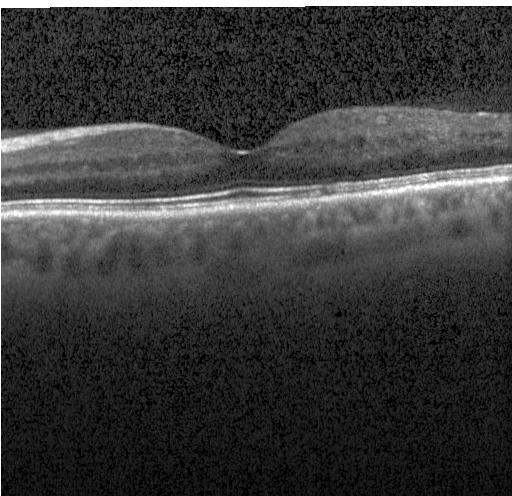
OCT scan showing no choroidal neovascularization, no diabetic macular edema, and no drusen.